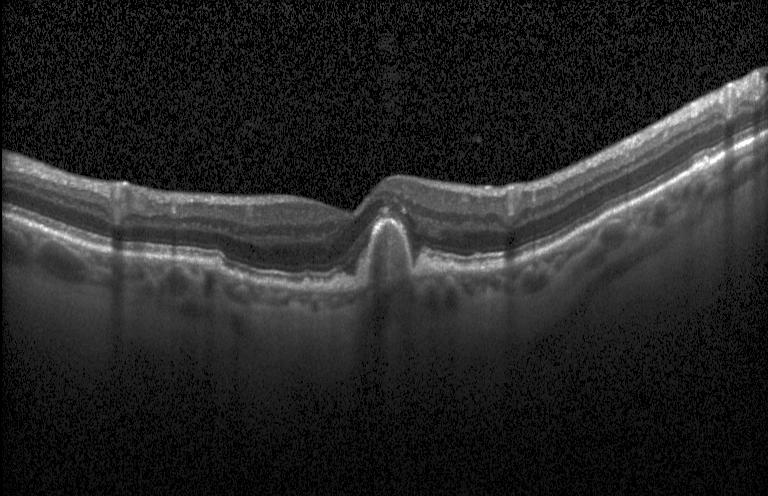 Sub-RPE drusenoid deposits.